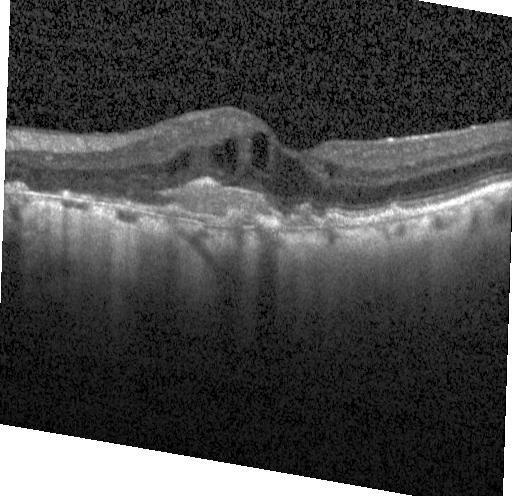

Heidelberg Spectralis OCT system, spectral-domain OCT, fovea-centered, optical coherence tomography scan. Assessment: choroidal neovascularization.